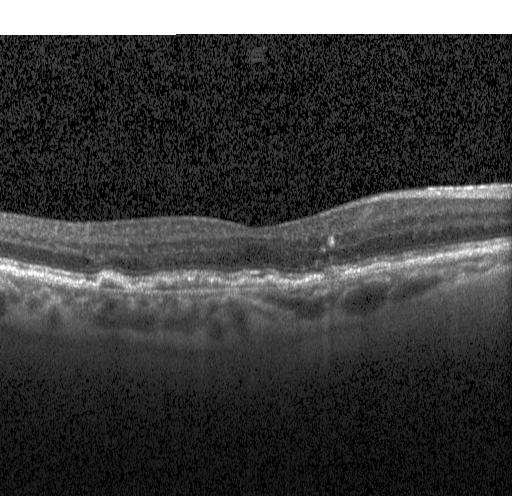
Through the macula · OCT B-scan · acquired on a Heidelberg Spectralis · spectral-domain optical coherence tomography.
Finding: a choroidal neovascular membrane.